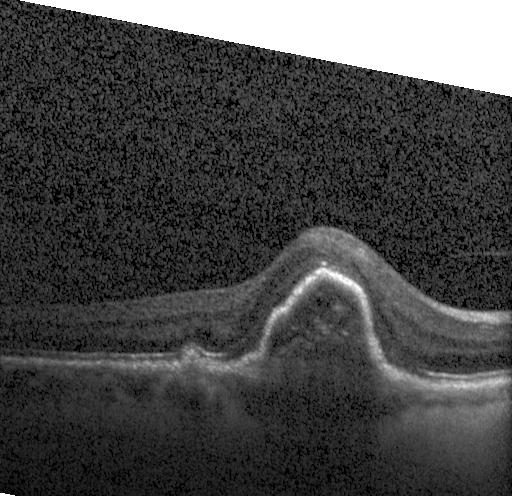

Heidelberg Spectralis, SD-OCT, optical coherence tomography scan, macular scan — This B-scan demonstrates choroidal neovascularization (CNV).